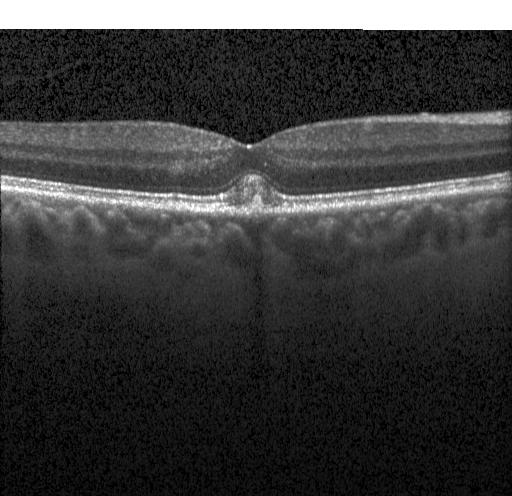 SD-OCT · OCT line scan · acquired on a Heidelberg Spectralis · horizontal scan through the fovea.
Finding: multiple drusen.